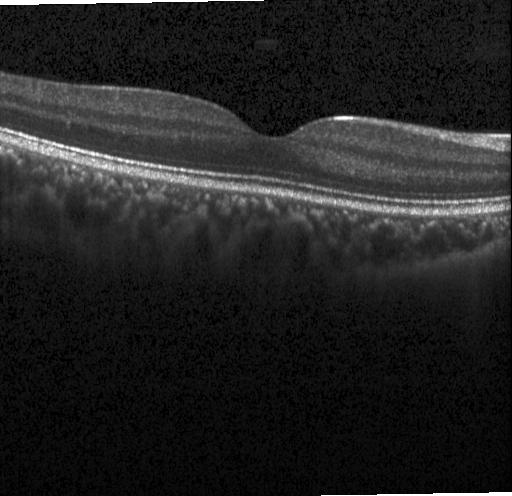
SD-OCT. Retinal OCT B-scan. Horizontal scan through the fovea. Instrument: Heidelberg Spectralis
This B-scan demonstrates no CNV, no DME, and no drusen.